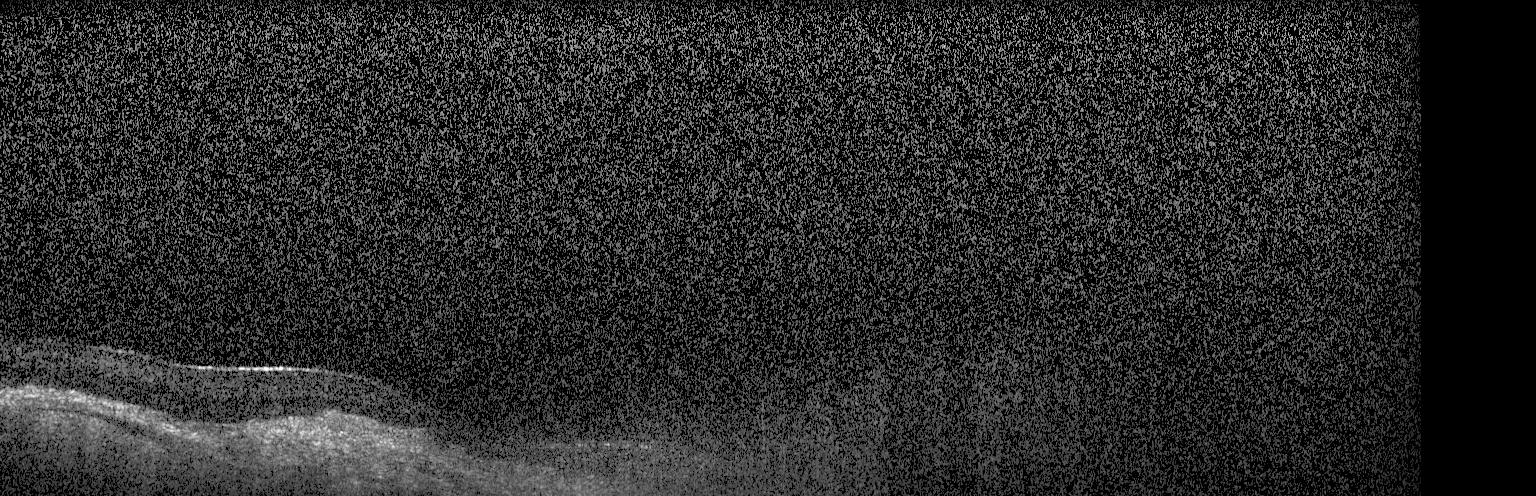
SD-OCT; retinal OCT cross-section
This B-scan demonstrates a choroidal neovascular membrane.